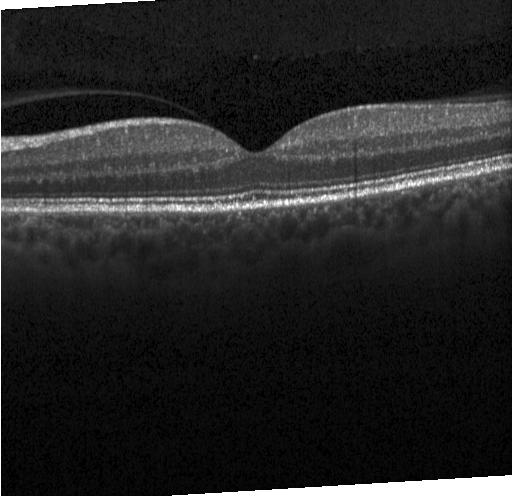
Spectral-domain optical coherence tomography · acquired on a Heidelberg Spectralis · macular scan · retinal OCT cross-section.
Impression: no choroidal neovascularization, no diabetic macular edema, and no drusen.